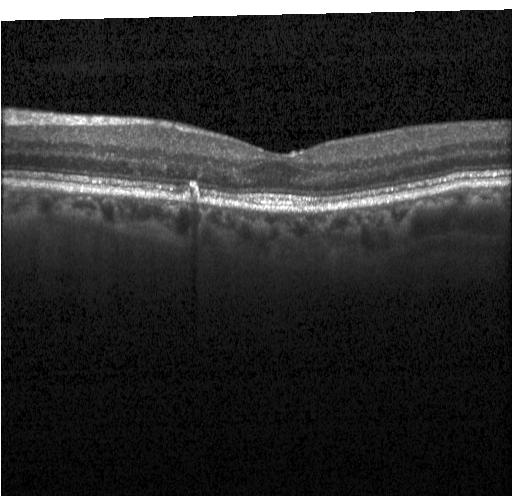 Macular OCT: multiple drusen.